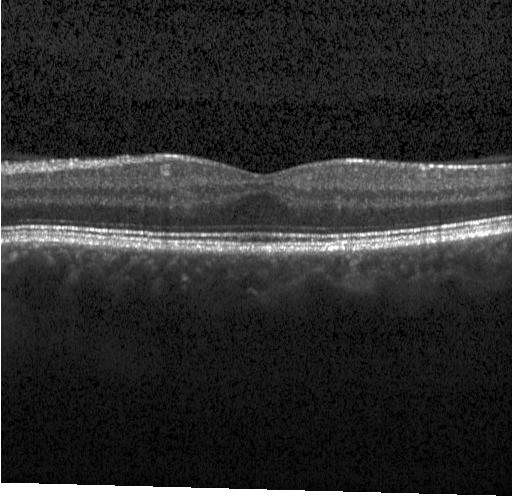

Fovea-centered · SD-OCT · Heidelberg Spectralis · retinal OCT B-scan.
Diagnosis: no choroidal neovascularization, no diabetic macular edema, and no drusen.